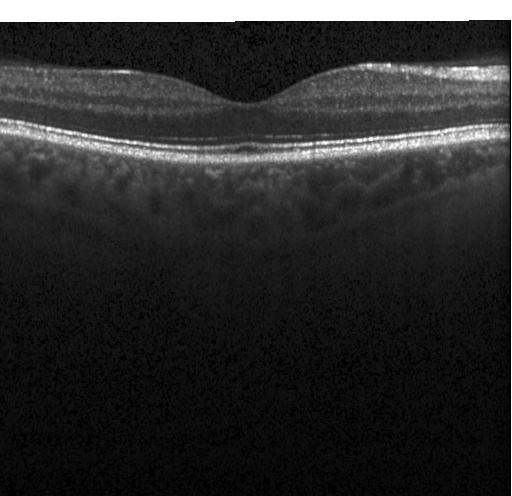 Optical coherence tomography scan; through the macula — No choroidal neovascularization, diabetic macular edema, or drusen.